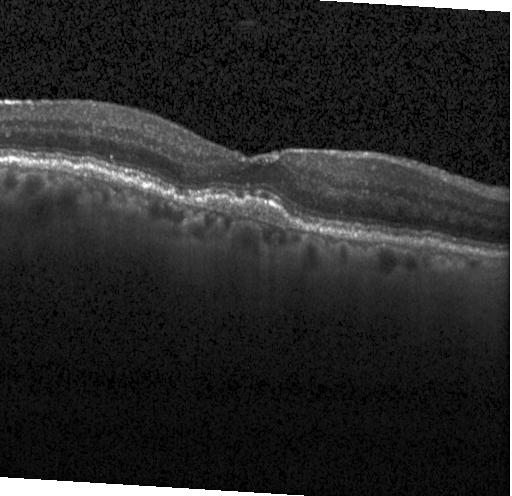
Spectral-domain OCT; OCT line scan. OCT finding: a choroidal neovascular membrane.